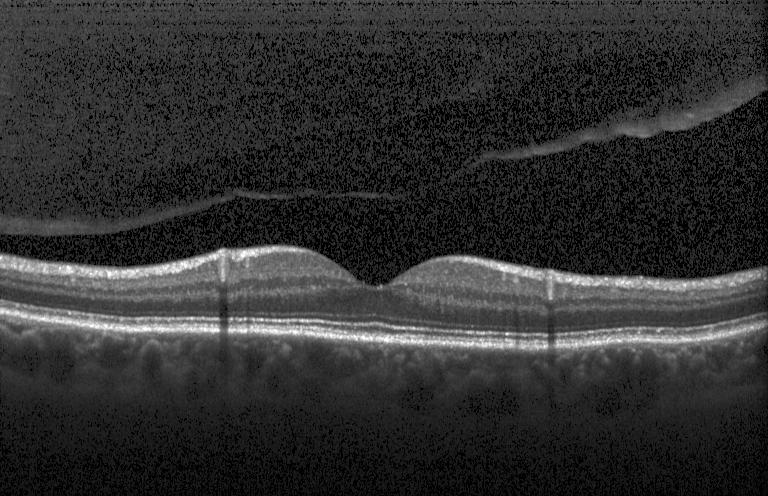
Assessment: no choroidal neovascularization, no diabetic macular edema, and no drusen.